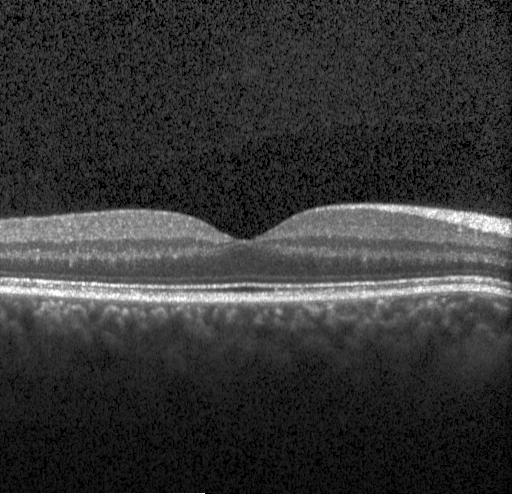

Assessment: no choroidal neovascularization, diabetic macular edema, or drusen.